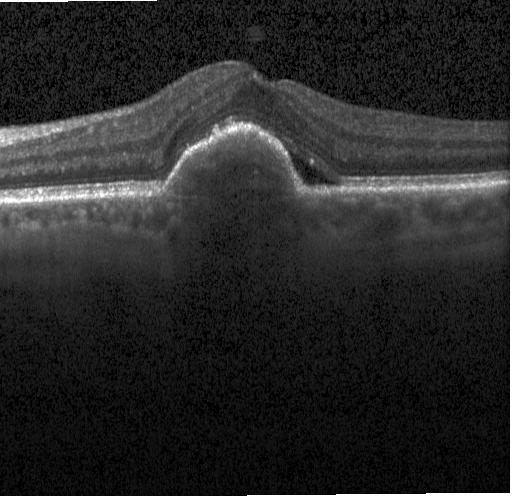

Dx: choroidal neovascularization (CNV).